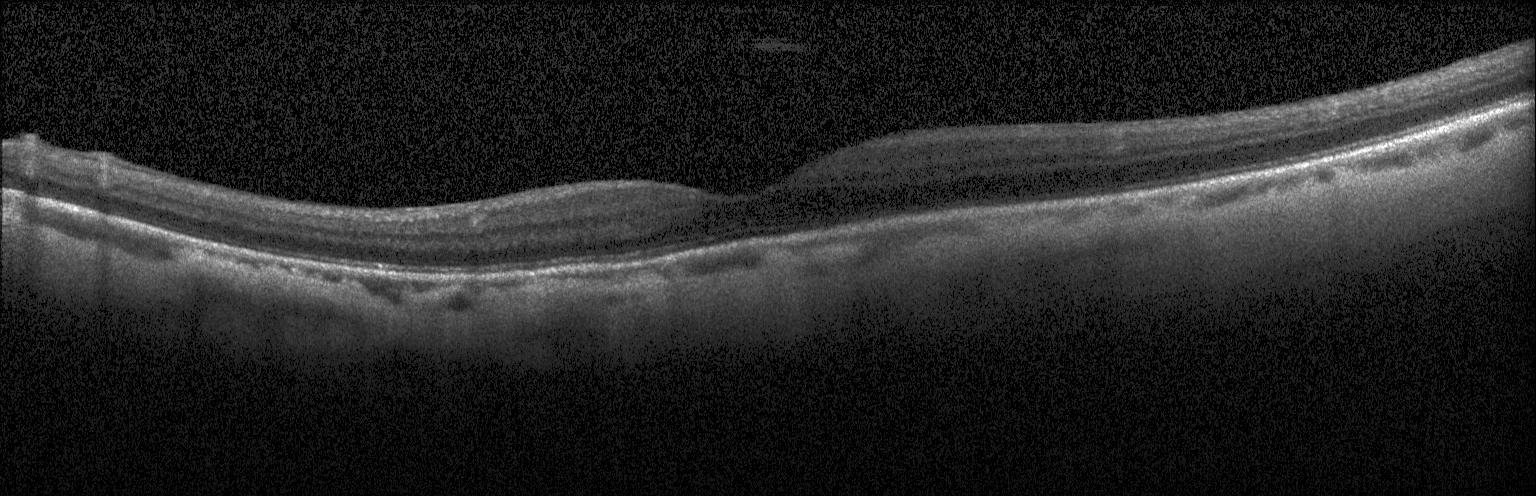 Dx: no CNV, no DME, and no drusen.